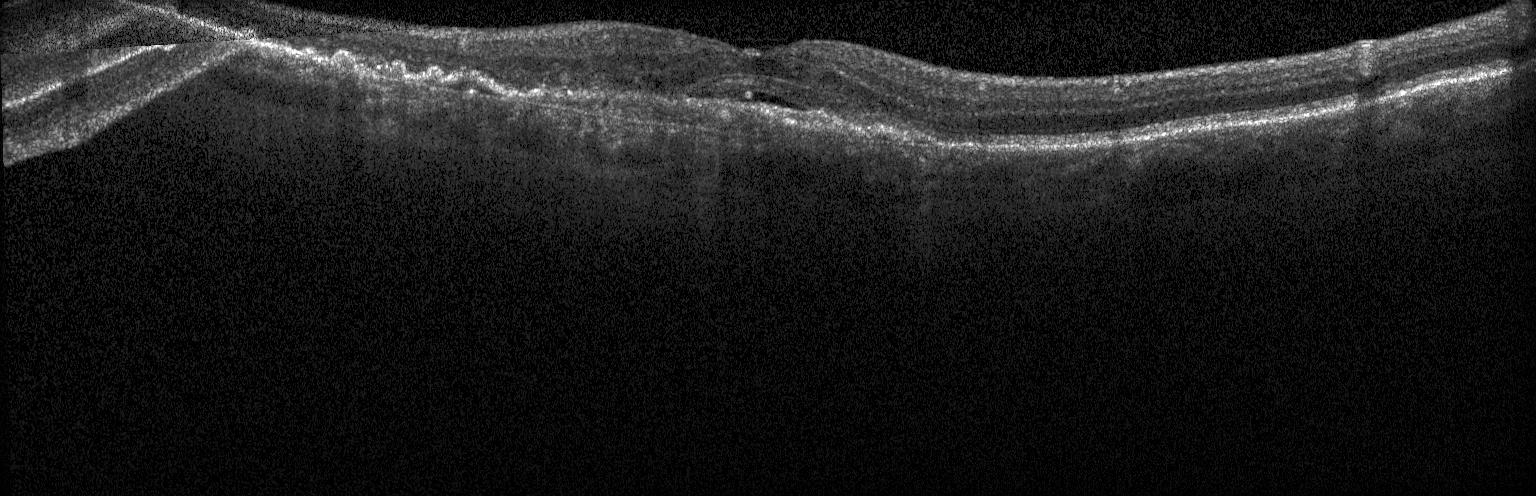

OCT finding: a choroidal neovascular membrane.